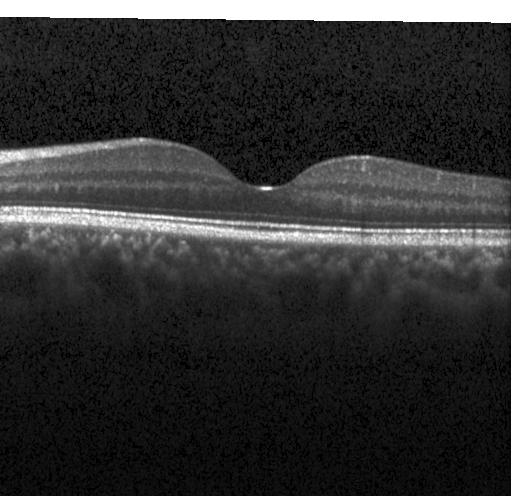

Macular OCT demonstrating no evidence of choroidal neovascularization, diabetic macular edema, or drusen.